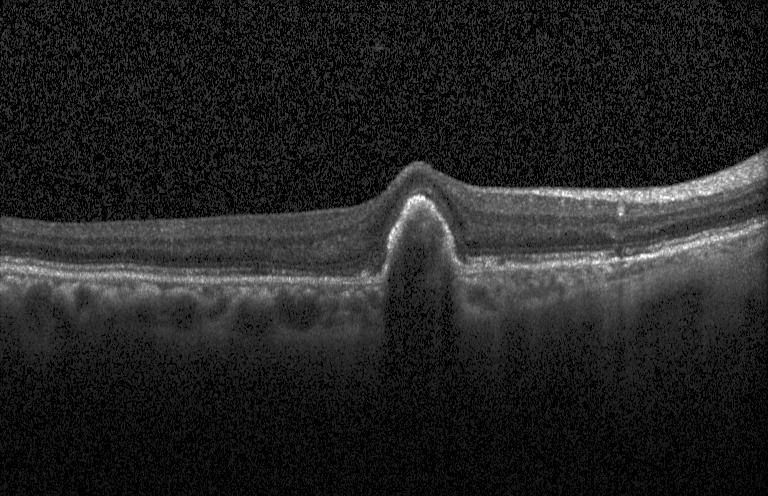
OCT finding: a choroidal neovascular membrane.